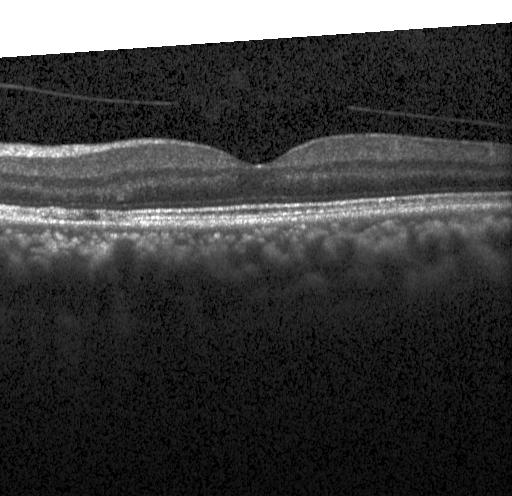 Spectral-domain OCT; optical coherence tomography B-scan; acquired on a Heidelberg Spectralis; centered on the fovea
Diagnosis: no choroidal neovascularization, no diabetic macular edema, and no drusen.